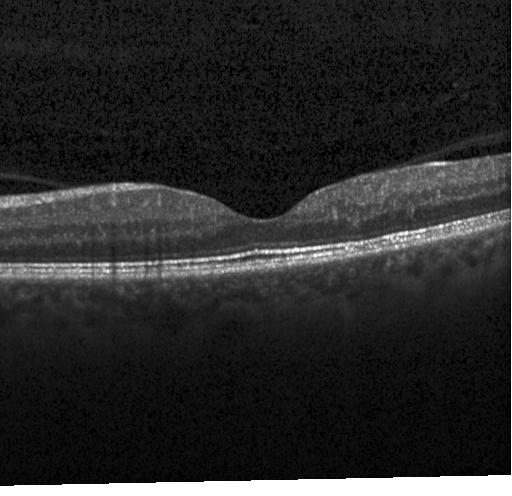
Retinal OCT B-scan, instrument: Heidelberg Spectralis, spectral-domain OCT
Impression: neither choroidal neovascularization, diabetic macular edema, nor drusen.